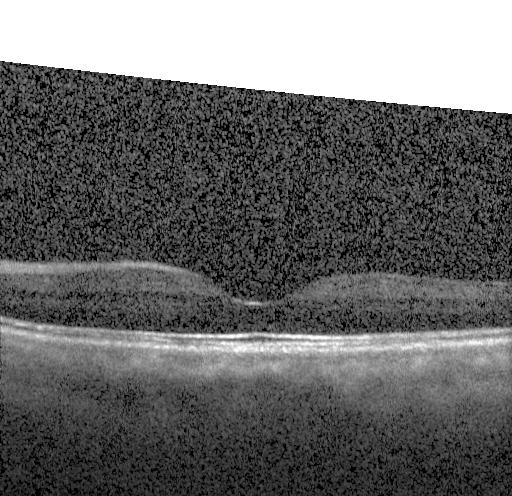
Retinal OCT cross-section. Instrument: Heidelberg Spectralis — Dx: no choroidal neovascularization, diabetic macular edema, or drusen.